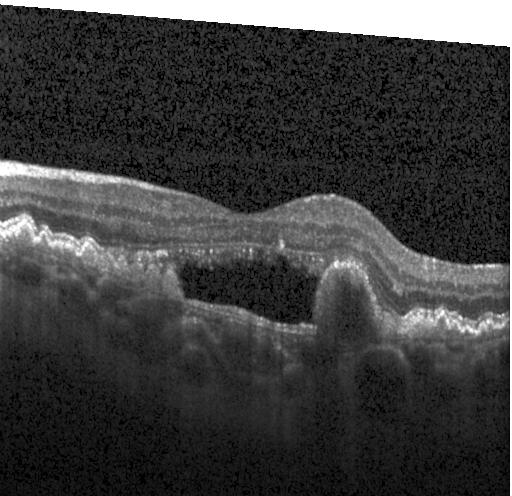

Optical coherence tomography B-scan. Diagnosis: a choroidal neovascular membrane.